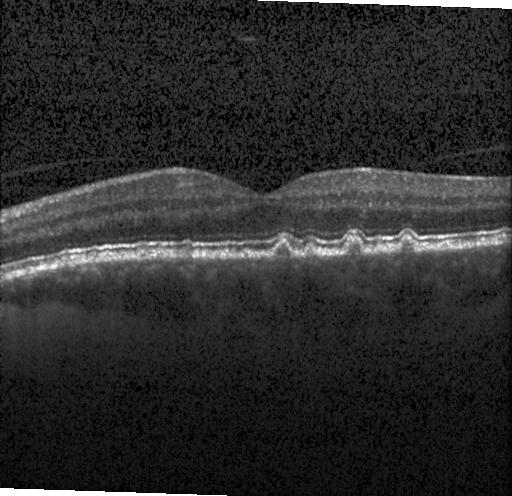

Diagnosis: drusen.